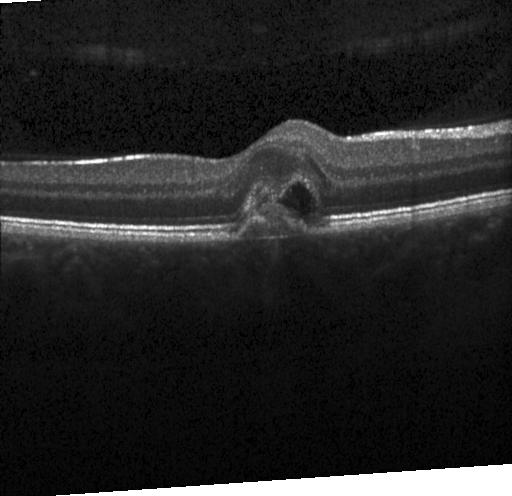 OCT line scan — Finding: choroidal neovascularization.